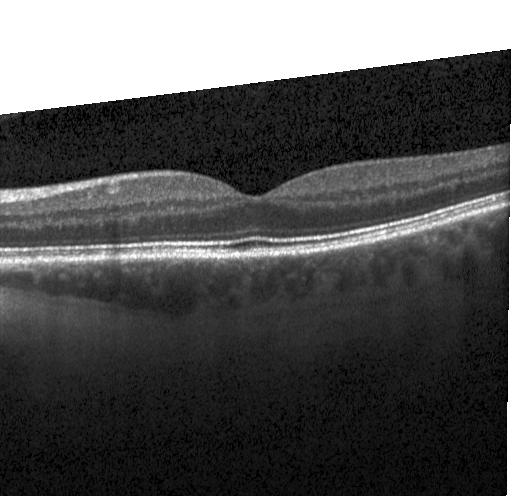

Macular OCT demonstrating no CNV, no DME, and no drusen.